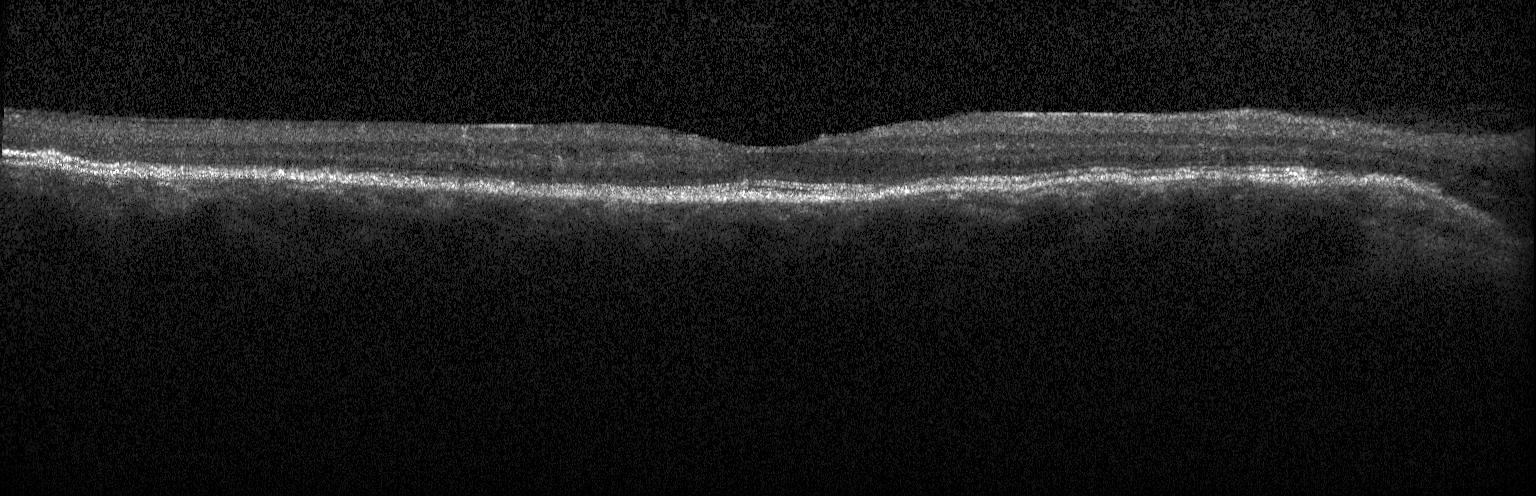

Dx: no CNV, no DME, and no drusen.